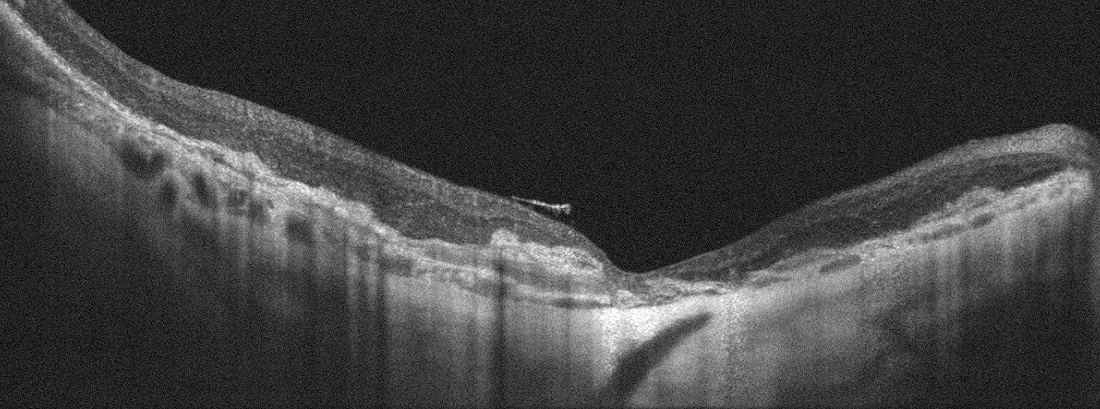
OCT B-scan showing AMD.